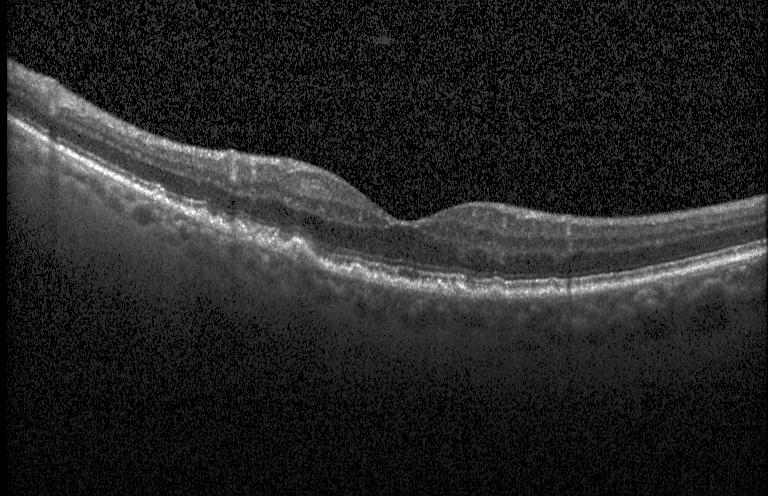 Horizontal scan through the fovea. Spectral-domain OCT. Retinal OCT B-scan
Impression: drusen.